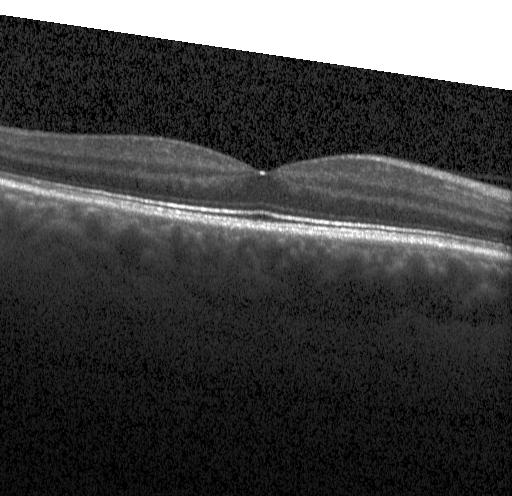

Fovea-centered, SD-OCT, instrument: Heidelberg Spectralis, optical coherence tomography B-scan
Neither CNV, DME, nor drusen.